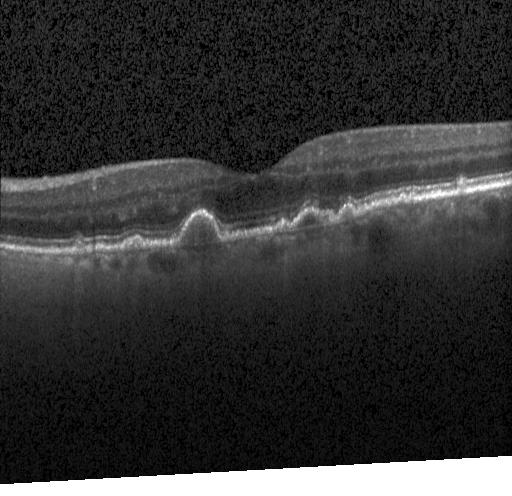 Finding: drusen.